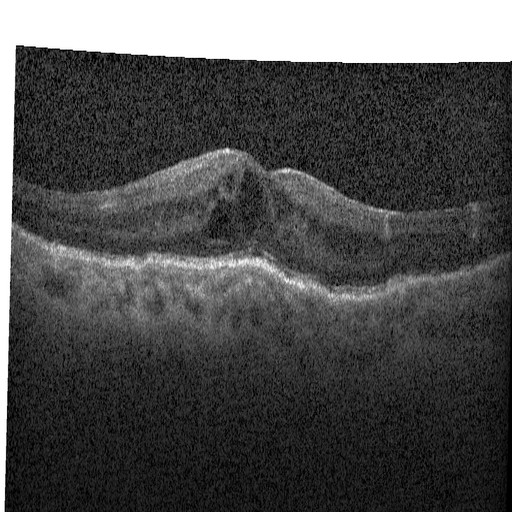 Heidelberg Spectralis OCT system. Through the macula. Retinal OCT cross-section
Macular OCT: diabetic macular edema (DME).